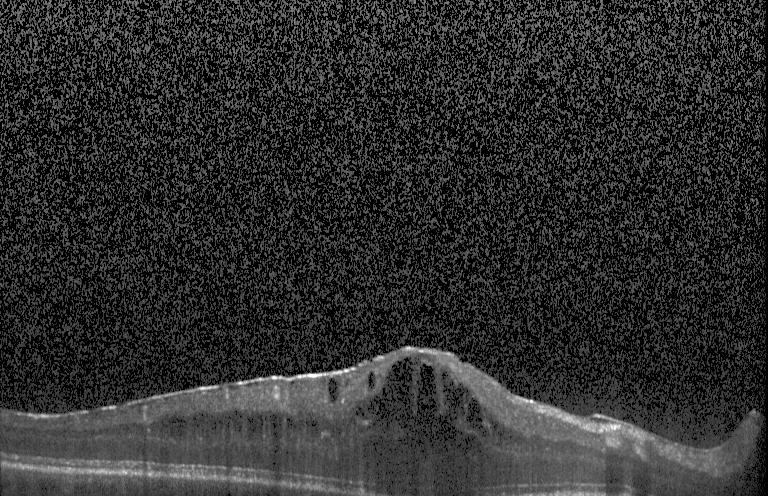 OCT B-scan; SD-OCT; centered on the fovea
OCT finding: diabetic macular edema.